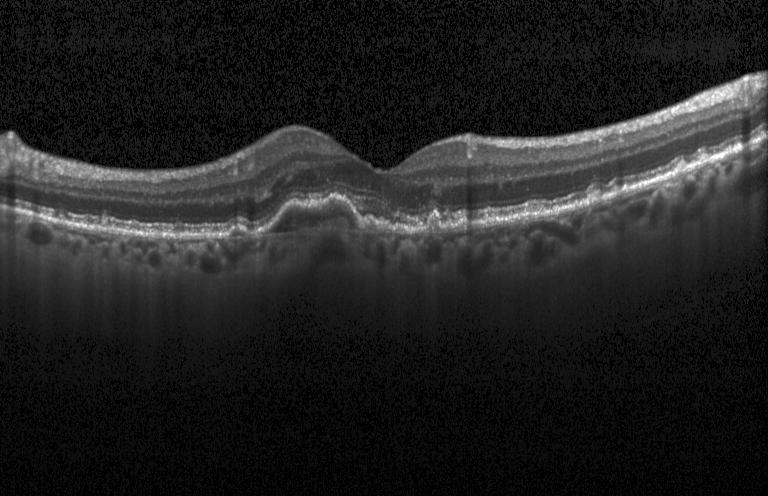 Impression: choroidal neovascularization.